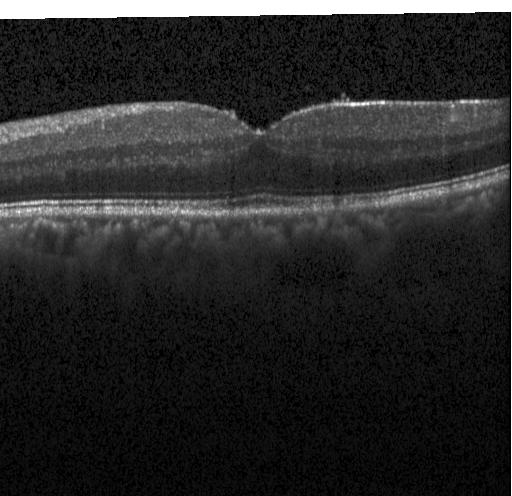 Instrument: Heidelberg Spectralis. Horizontal scan through the fovea. SD-OCT. Optical coherence tomography scan. Diagnosis: no evidence of choroidal neovascularization, diabetic macular edema, or drusen.